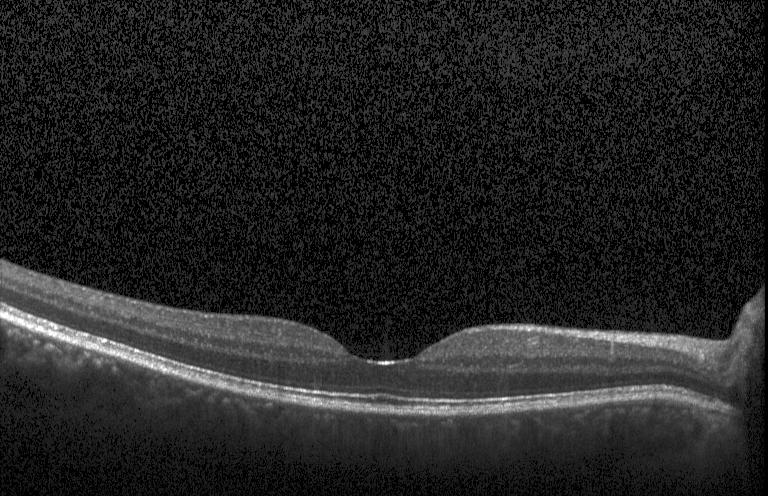

Optical coherence tomography scan; instrument: Heidelberg Spectralis
Finding: no evidence of choroidal neovascularization, diabetic macular edema, or drusen.